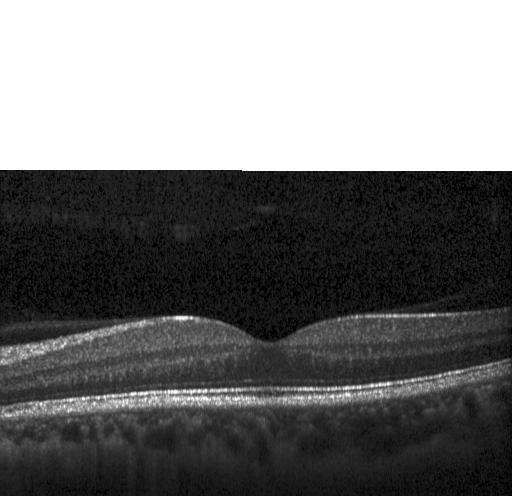
Impression: no choroidal neovascularization, no diabetic macular edema, and no drusen.